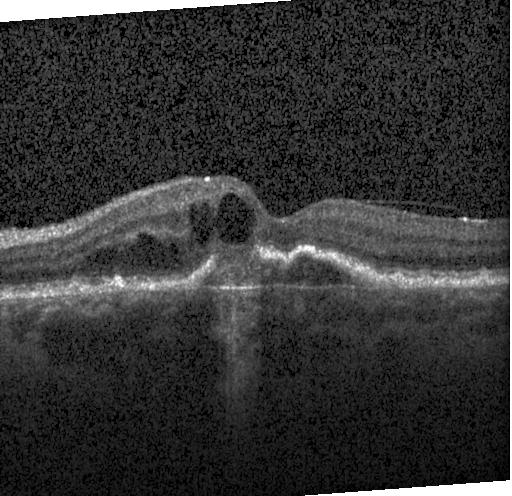 Retinal OCT B-scan
Finding: CNV.